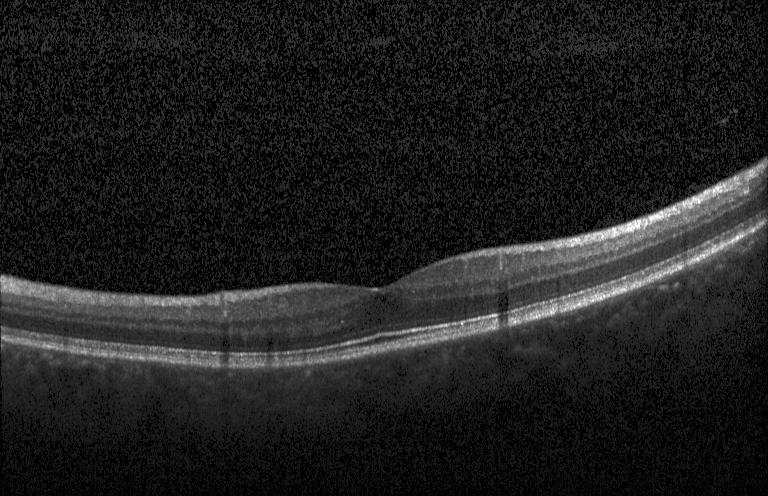 Through the macula. Heidelberg Spectralis OCT system. Spectral-domain OCT. OCT line scan. Finding: no choroidal neovascularization, no diabetic macular edema, and no drusen.